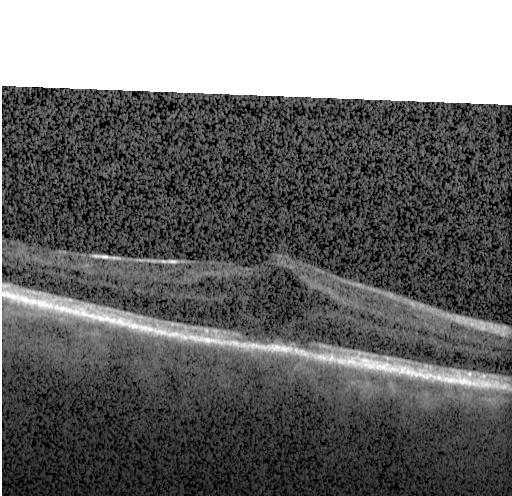 Through the macula. Spectral-domain optical coherence tomography. Retinal OCT cross-section — Finding: diabetic macular edema (DME).